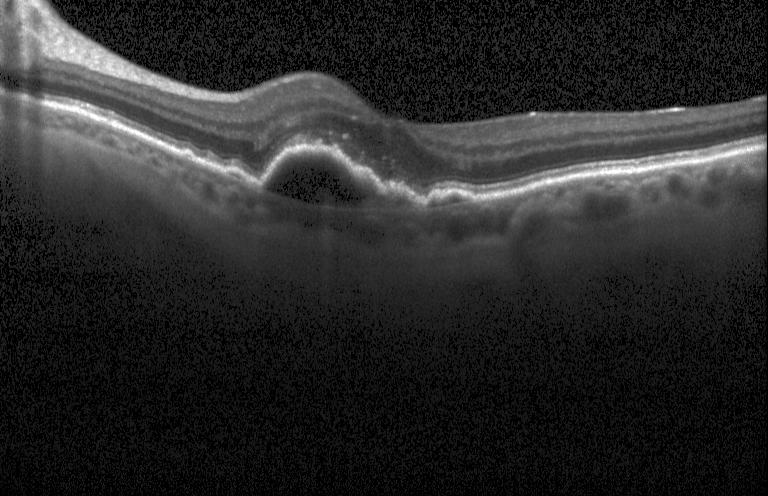
Macular OCT demonstrating choroidal neovascularization.